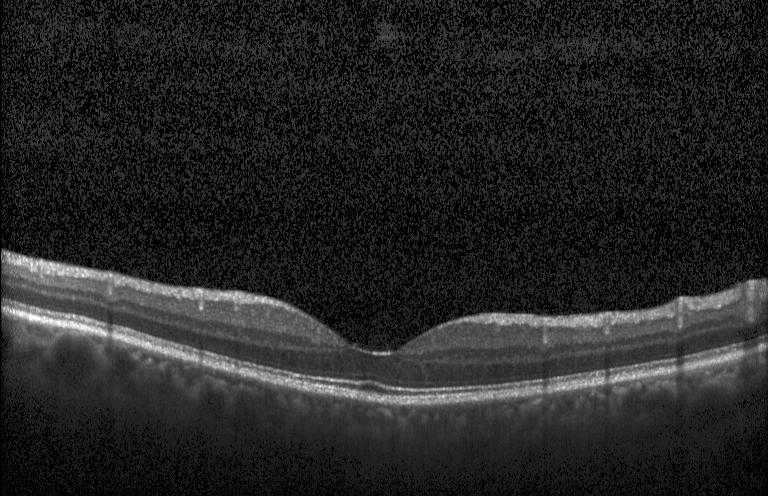
Diagnosis: neither CNV, DME, nor drusen.